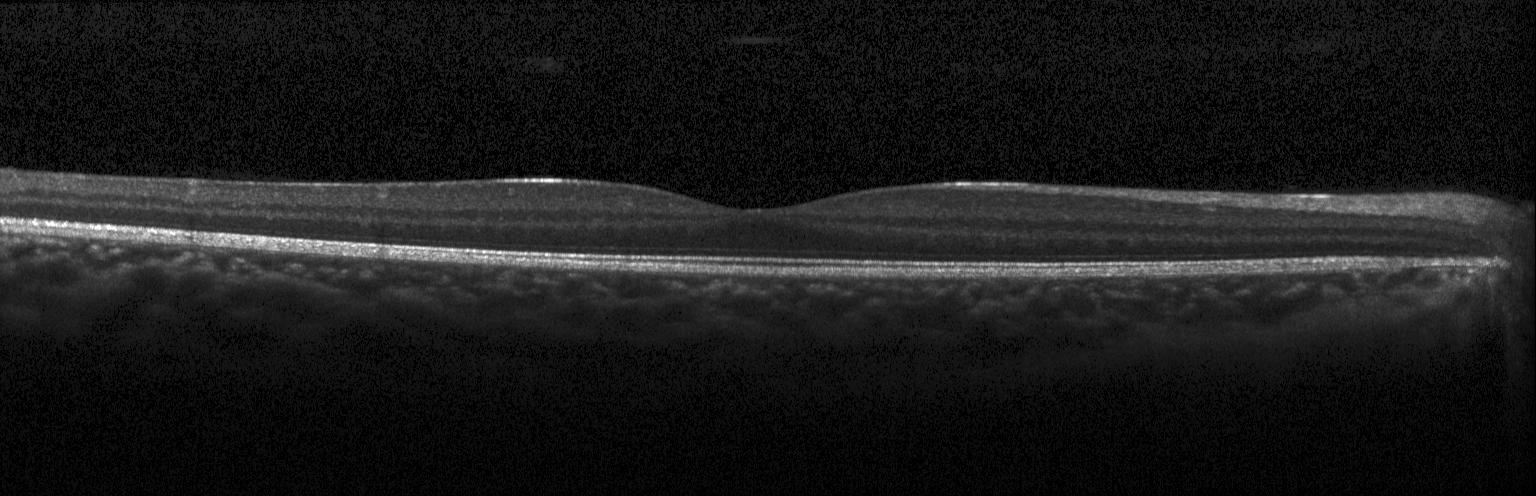 Retinal OCT B-scan
Assessment: no evidence of CNV, DME, or drusen.